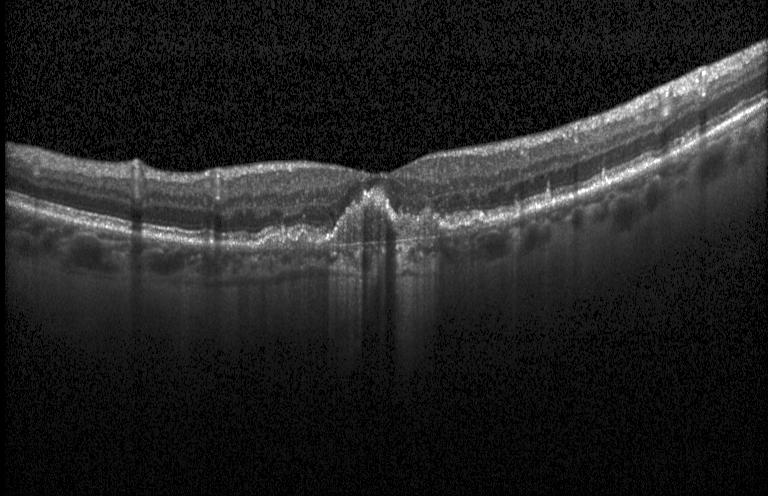 Diagnosis: a choroidal neovascular membrane.